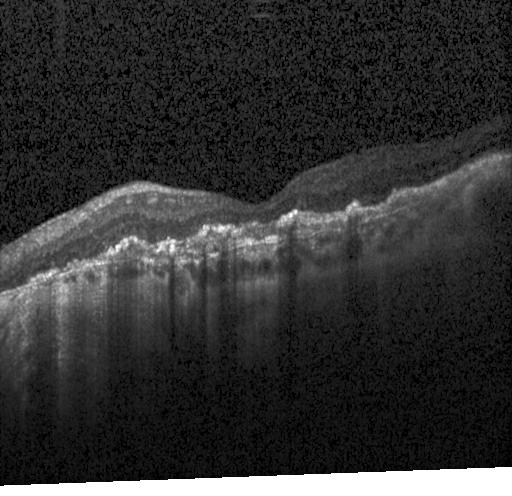
Diagnosis: a choroidal neovascular membrane.